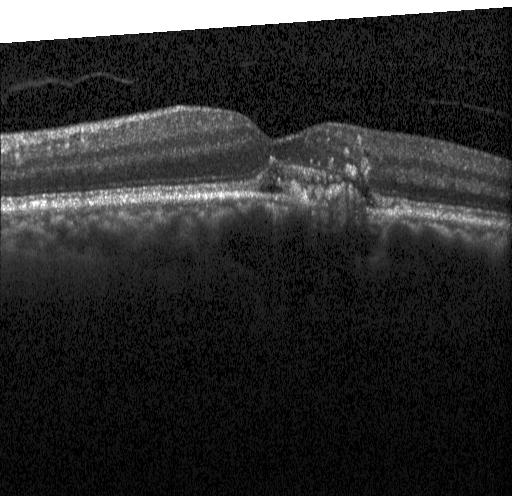

Spectral-domain OCT B-scan: choroidal neovascularization (CNV).